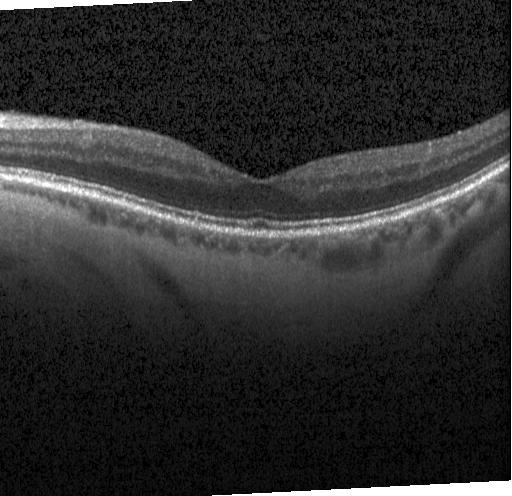 SD-OCT · retinal OCT cross-section · instrument: Heidelberg Spectralis · horizontal scan through the fovea.
No CNV, DME, or drusen.